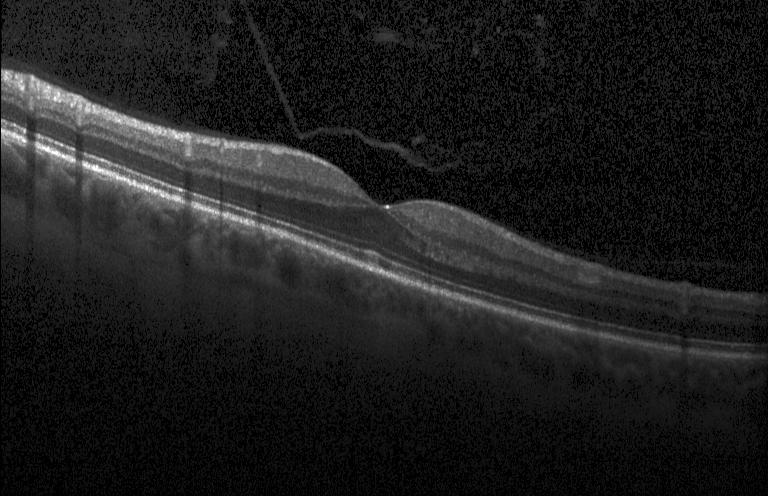 Acquired on a Heidelberg Spectralis. SD-OCT. OCT line scan.
Diagnosis: no evidence of choroidal neovascularization, diabetic macular edema, or drusen.